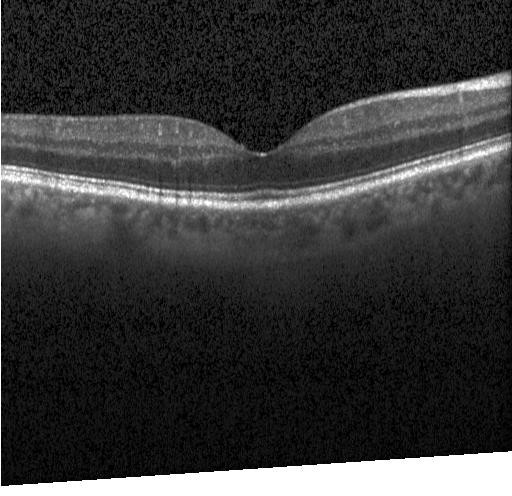
OCT B-scan
OCT finding: no evidence of choroidal neovascularization, diabetic macular edema, or drusen.